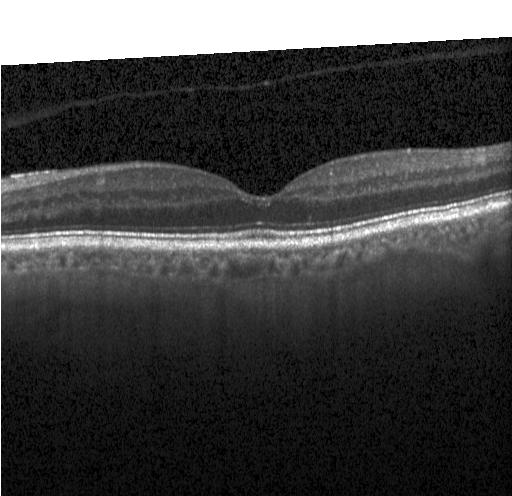
OCT scan showing no choroidal neovascularization, diabetic macular edema, or drusen.